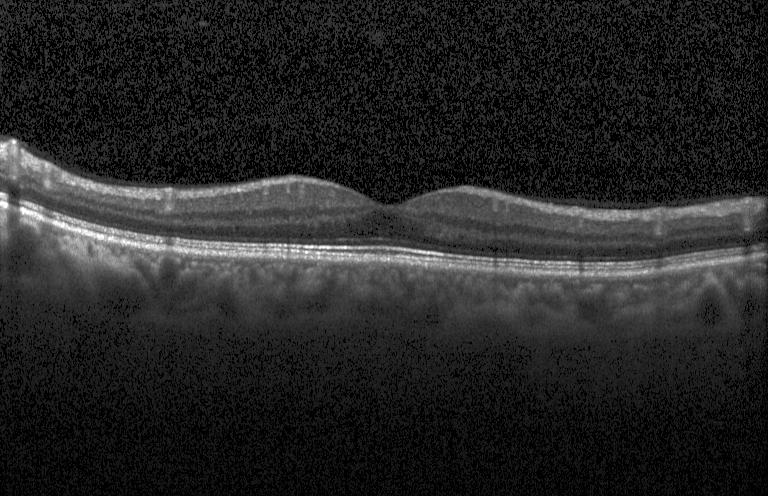
Dx: neither choroidal neovascularization, diabetic macular edema, nor drusen.